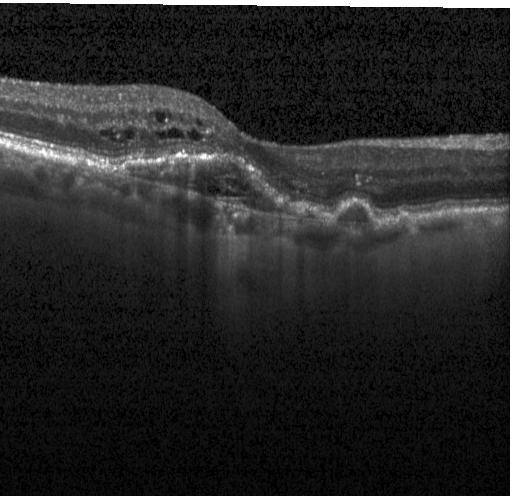

SD-OCT, optical coherence tomography scan. Assessment: a choroidal neovascular membrane.